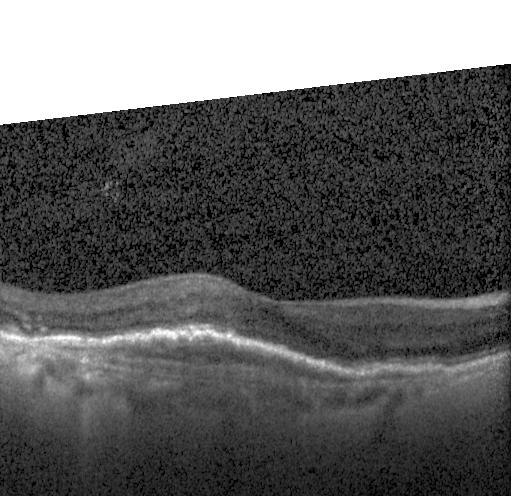 OCT finding: a choroidal neovascular membrane.